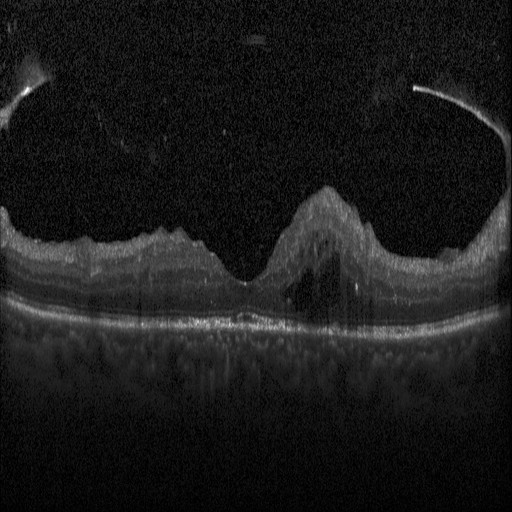 Spectral-domain optical coherence tomography. Retinal OCT B-scan. Heidelberg Spectralis. Centered on the fovea — Diagnosis: diabetic macular edema (DME).